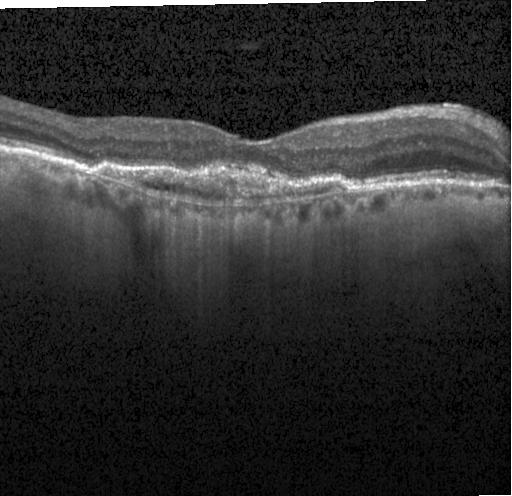
A choroidal neovascular membrane.